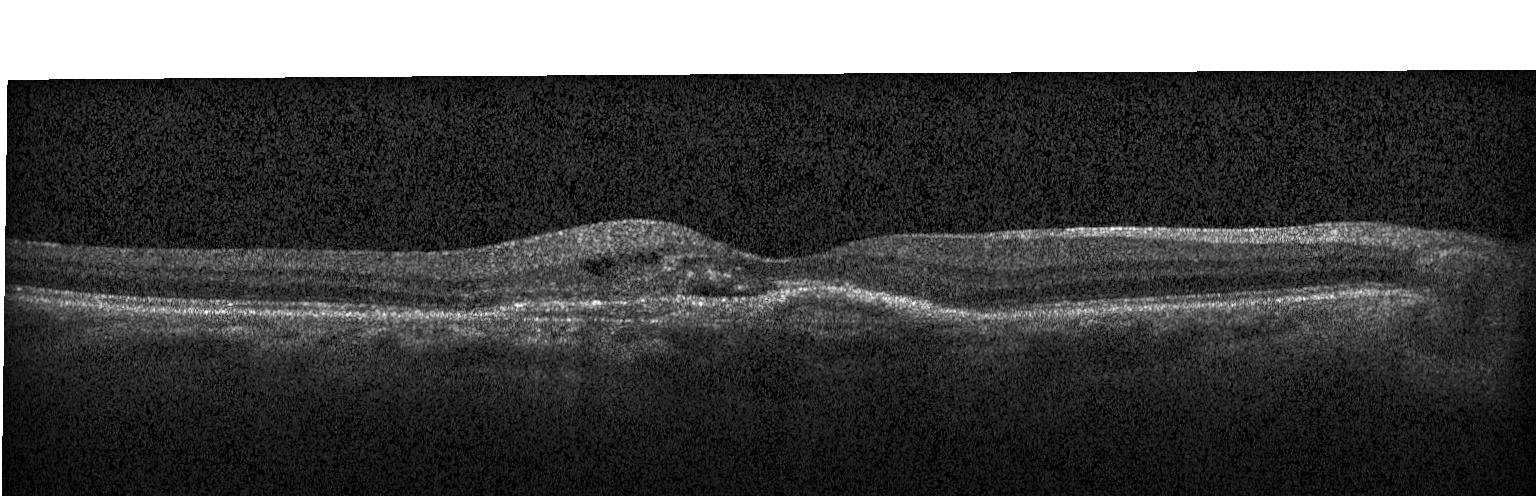 Through the macula. Retinal OCT cross-section. Acquired on a Heidelberg Spectralis. SD-OCT — Impression: choroidal neovascularization.